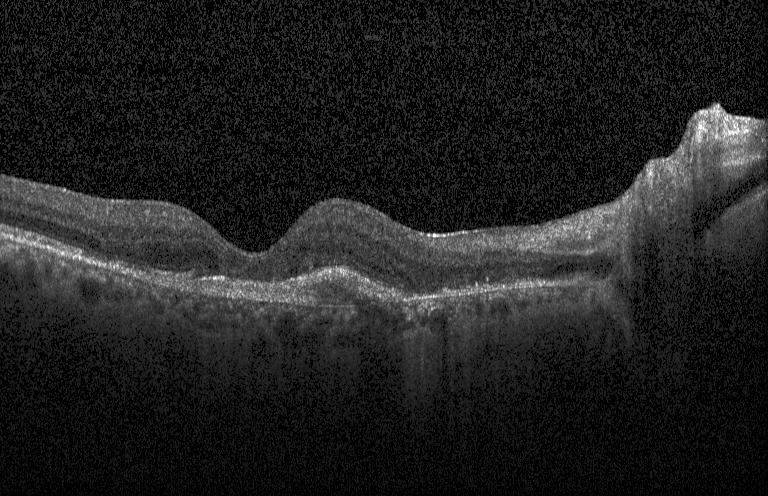
Centered on the fovea · OCT line scan · Heidelberg Spectralis
A choroidal neovascular membrane.